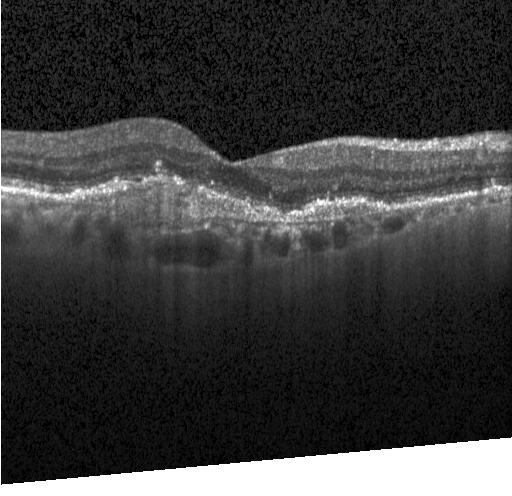 Heidelberg Spectralis · spectral-domain OCT · retinal OCT B-scan · through the macula.
Impression: a choroidal neovascular membrane.